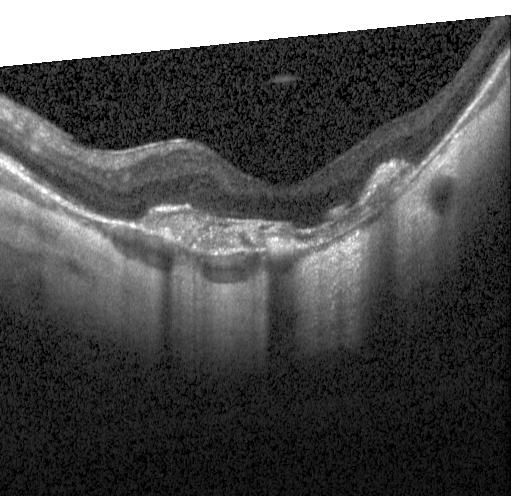
Spectral-domain OCT B-scan: choroidal neovascularization (CNV).